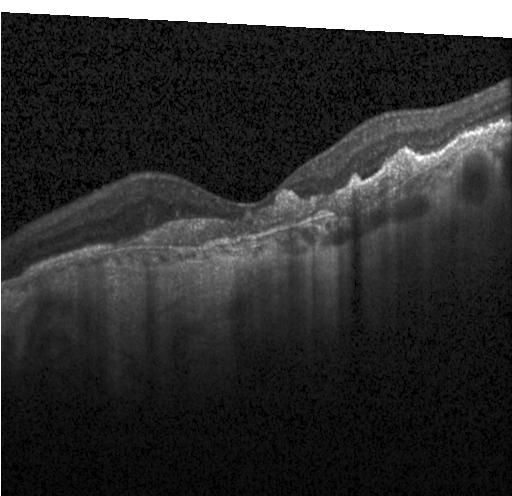 Instrument: Heidelberg Spectralis, through the macula, optical coherence tomography scan.
Diagnosis: a choroidal neovascular membrane.